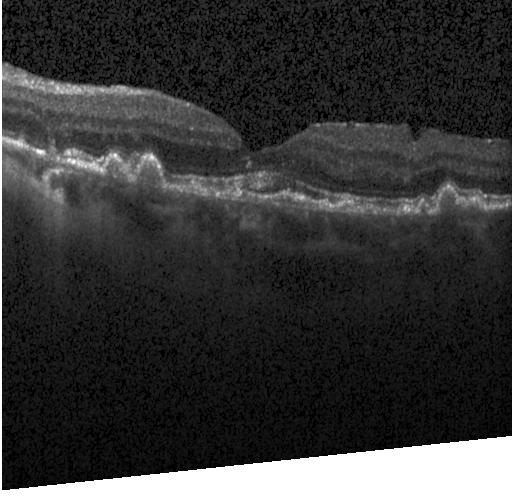

OCT B-scan, through the macula, instrument: Heidelberg Spectralis, spectral-domain OCT
Impression: choroidal neovascularization.